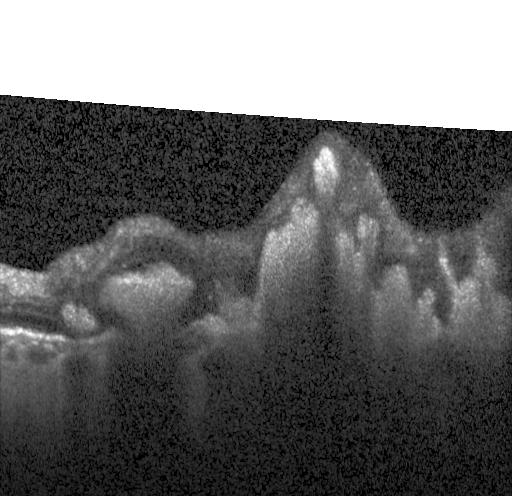

Macular scan · Heidelberg Spectralis OCT system · optical coherence tomography B-scan. Choroidal neovascularization.